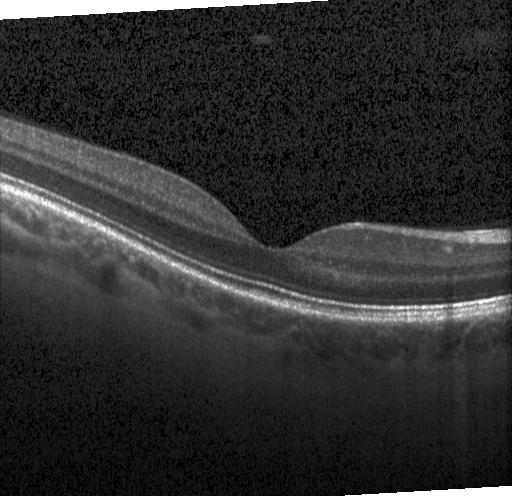

Finding: no evidence of CNV, DME, or drusen.